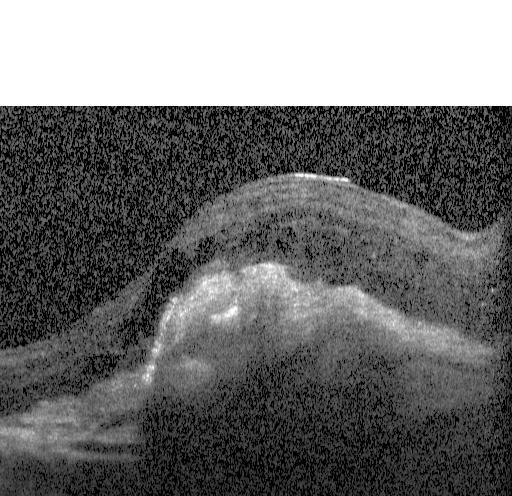

Assessment: a choroidal neovascular membrane.